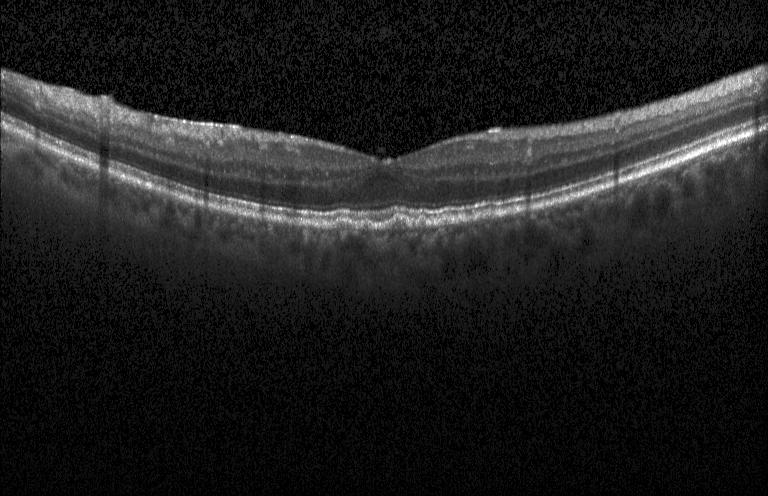 Retinal OCT cross-section
Diagnosis: sub-RPE drusenoid deposits.